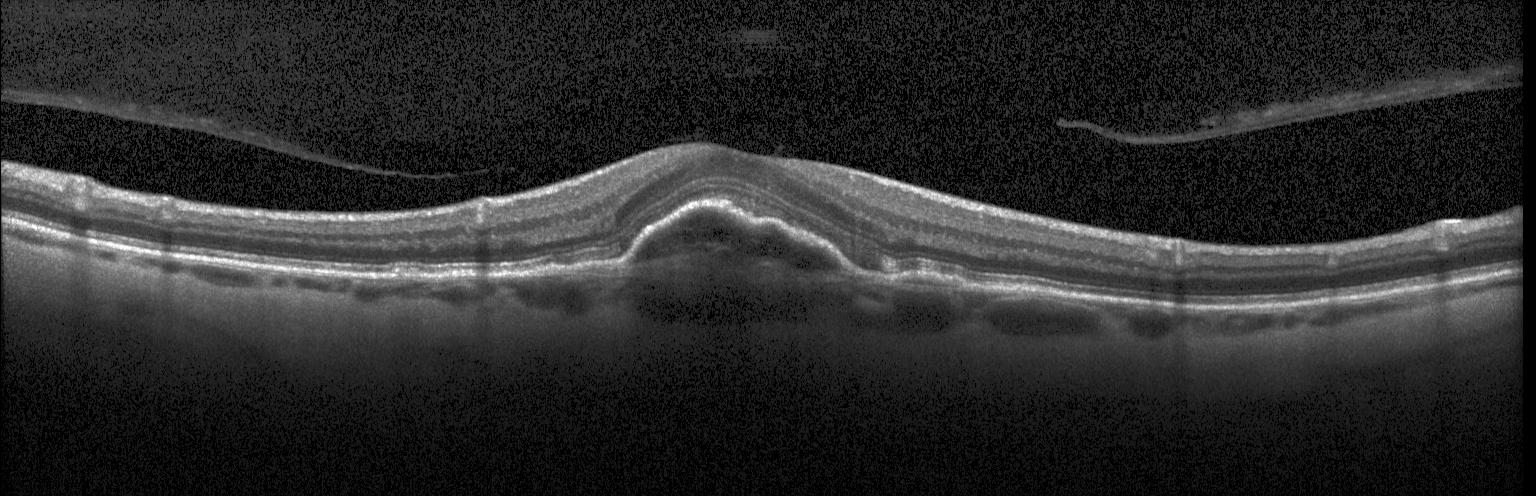

Macular OCT demonstrating choroidal neovascularization.